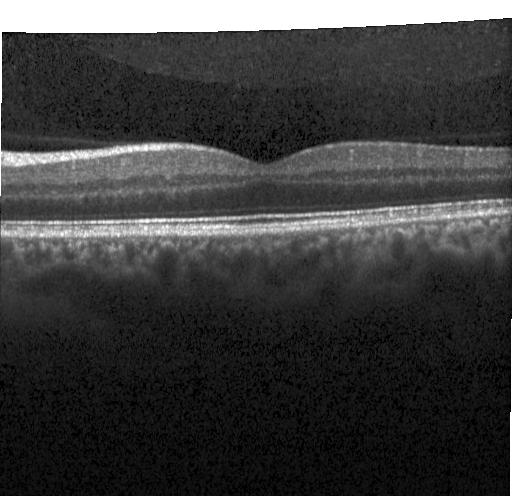
Retinal OCT cross-section. Horizontal scan through the fovea. Heidelberg Spectralis — Assessment: no CNV, no DME, and no drusen.